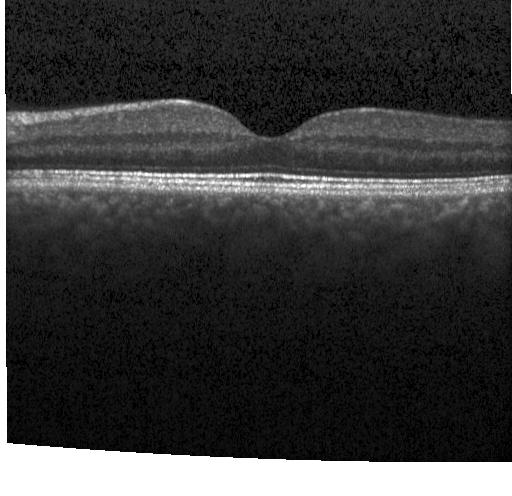

OCT line scan, spectral-domain optical coherence tomography, horizontal scan through the fovea — Assessment: no evidence of CNV, DME, or drusen.